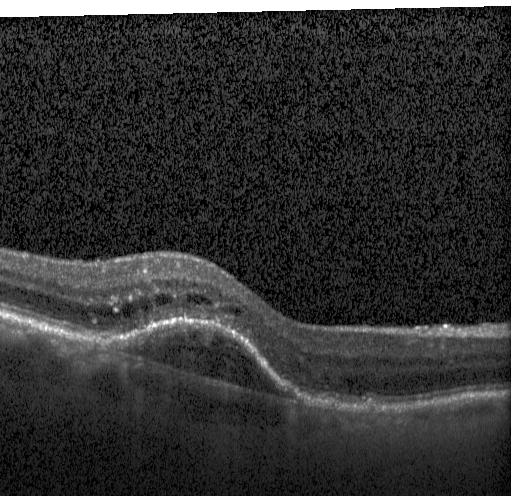 Retinal OCT cross-section, spectral-domain OCT, through the macula, acquired on a Heidelberg Spectralis. Diagnosis: choroidal neovascularization (CNV).